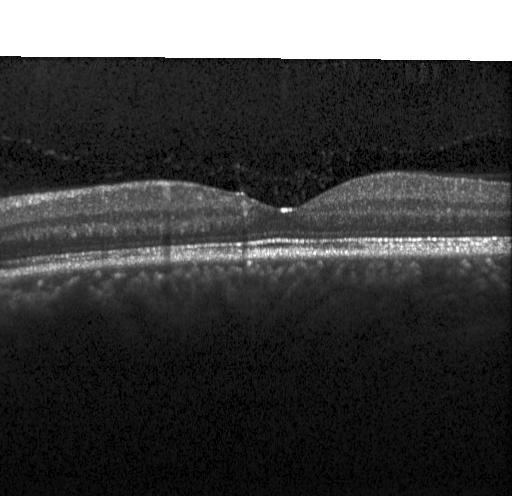

Macular OCT demonstrating neither choroidal neovascularization, diabetic macular edema, nor drusen.